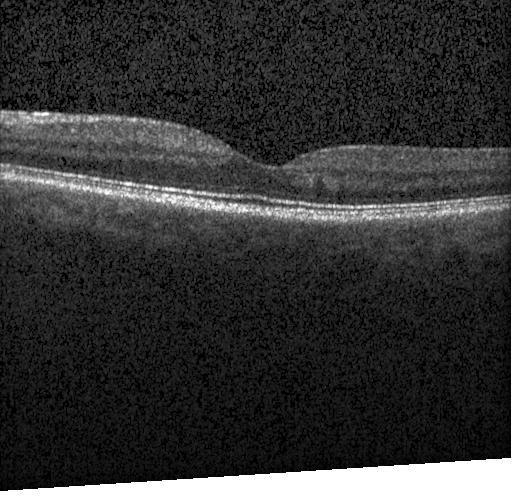

Assessment: no evidence of choroidal neovascularization, diabetic macular edema, or drusen.